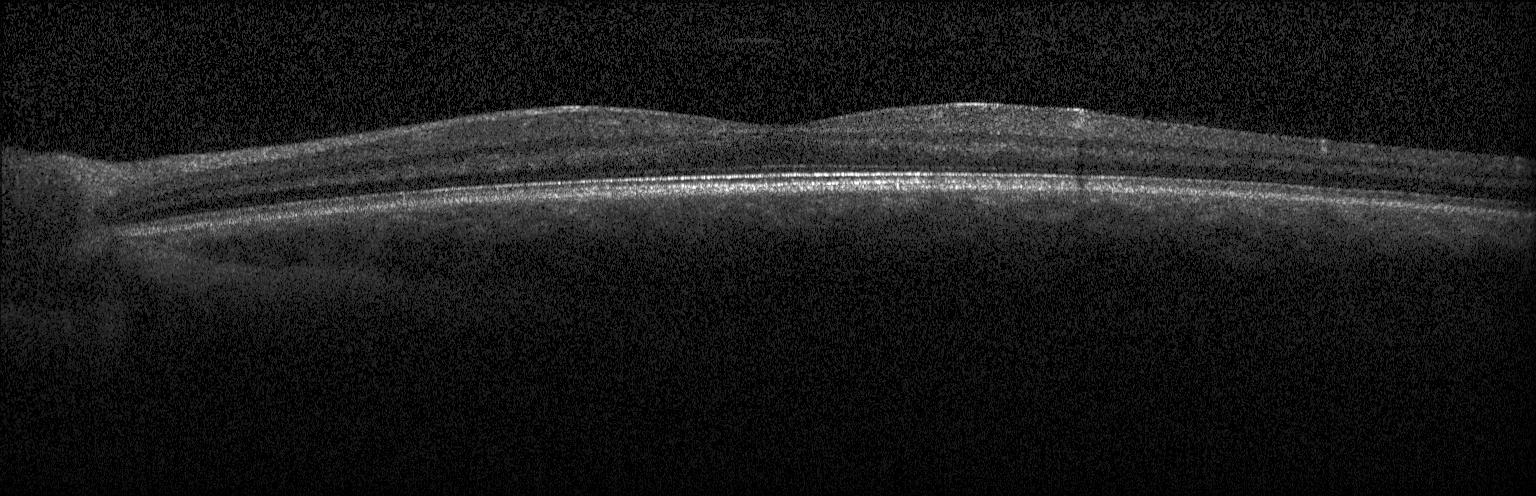

Macular OCT: no choroidal neovascularization, diabetic macular edema, or drusen.